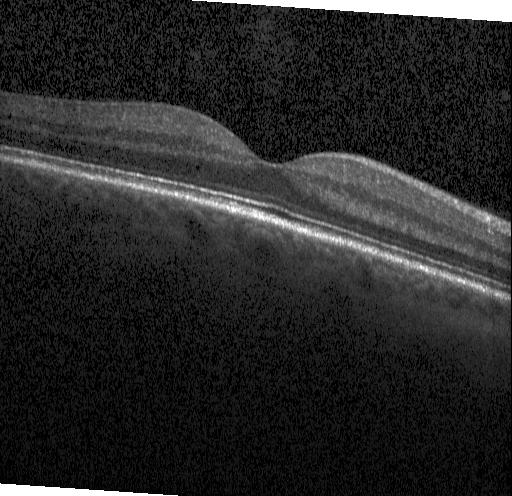

OCT scan showing no CNV, DME, or drusen.